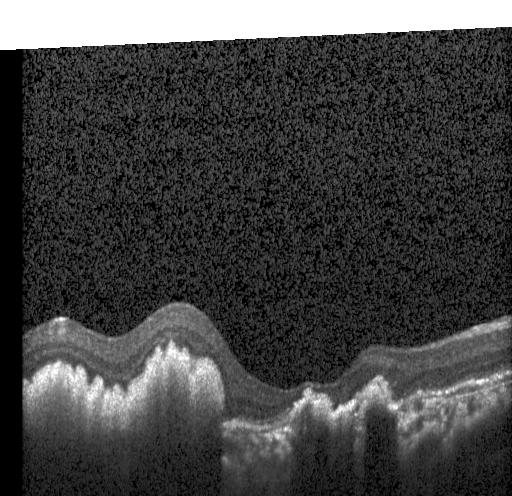

Spectral-domain OCT · retinal OCT cross-section · horizontal scan through the fovea. Finding: a choroidal neovascular membrane.